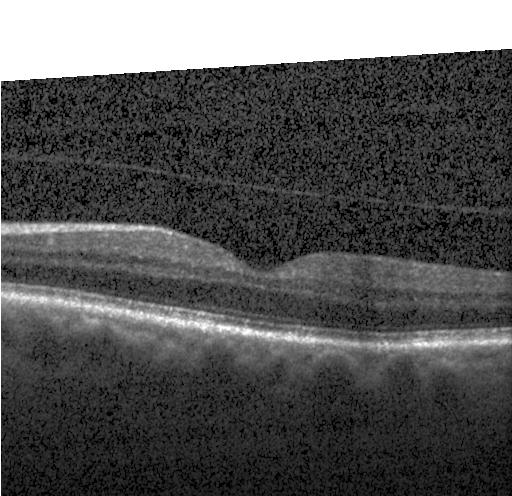 Finding: no choroidal neovascularization, no diabetic macular edema, and no drusen.